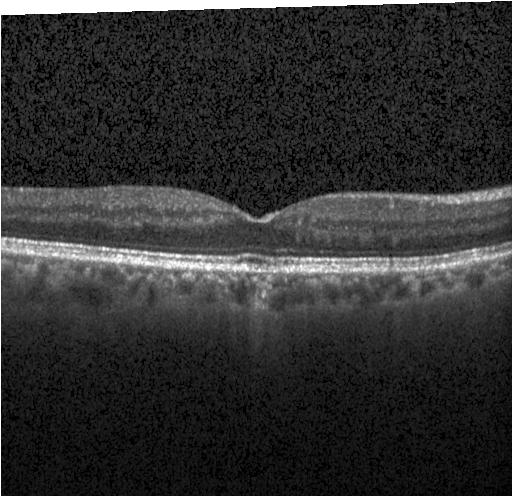
OCT B-scan showing no evidence of choroidal neovascularization, diabetic macular edema, or drusen.